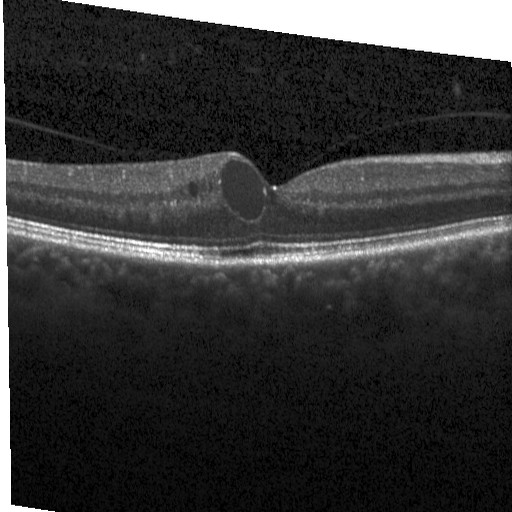

SD-OCT, centered on the fovea, acquired on a Heidelberg Spectralis, OCT line scan.
Finding: DME.